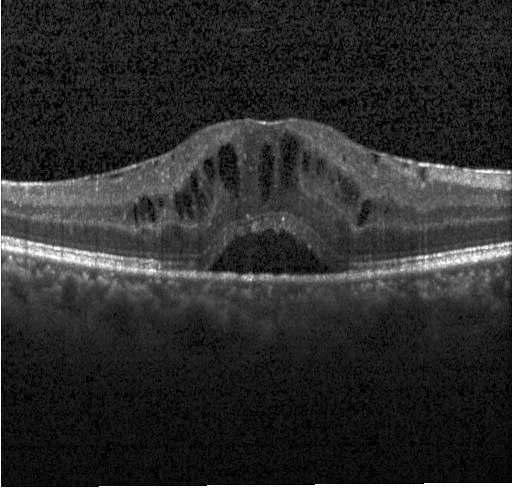

Spectral-domain optical coherence tomography. Optical coherence tomography B-scan. Heidelberg Spectralis OCT system. Fovea-centered — OCT finding: diabetic macular edema.